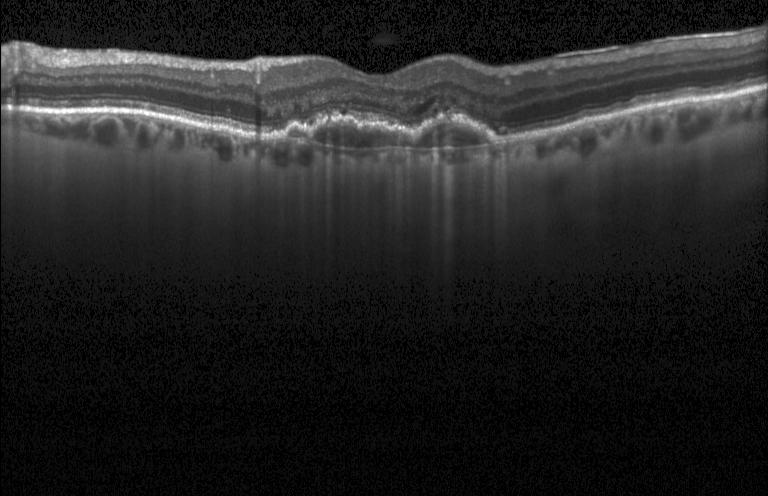 This B-scan demonstrates choroidal neovascularization.